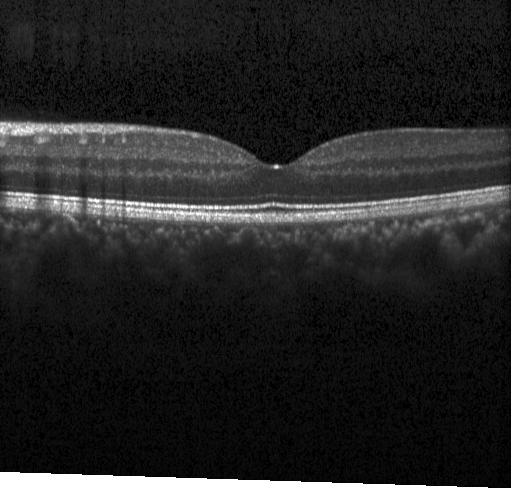
Diagnosis: no choroidal neovascularization, no diabetic macular edema, and no drusen.